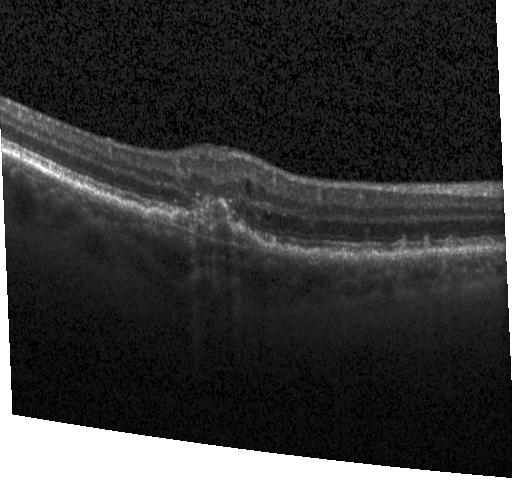 Centered on the fovea · retinal OCT cross-section · acquired on a Heidelberg Spectralis · spectral-domain OCT
Macular OCT: a choroidal neovascular membrane.